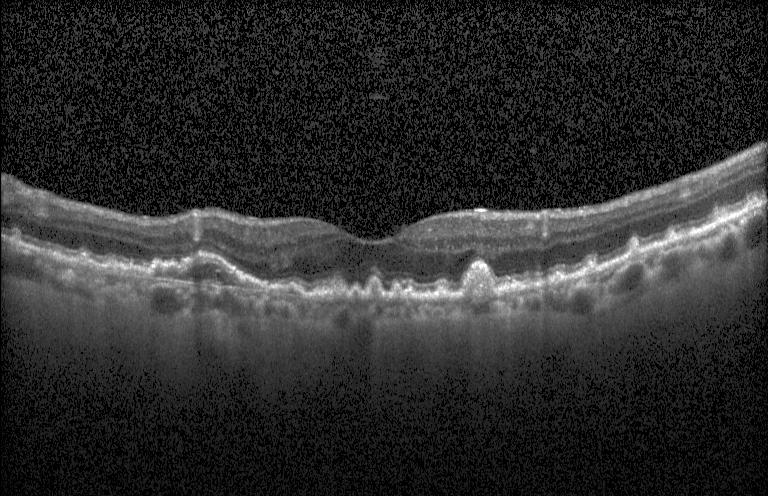
Multiple drusen.